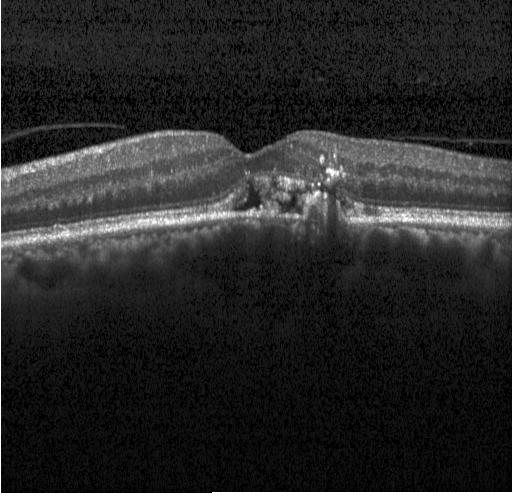
Centered on the fovea · SD-OCT · Heidelberg Spectralis OCT system · OCT line scan. CNV.